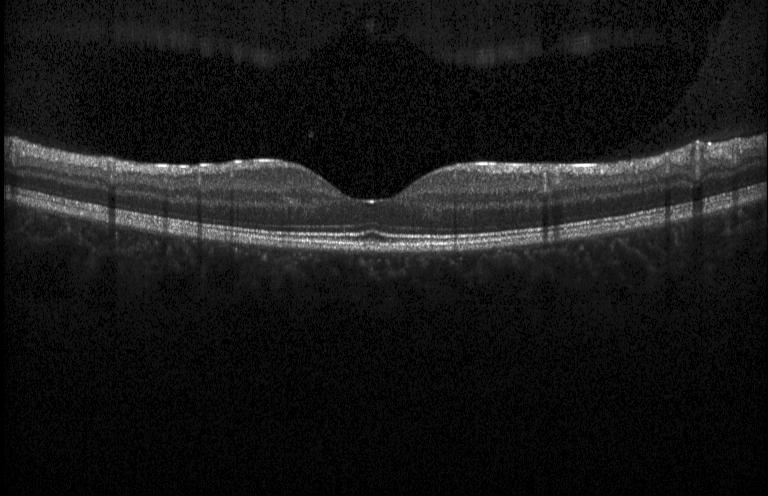
Retinal OCT cross-section showing no choroidal neovascularization, diabetic macular edema, or drusen.